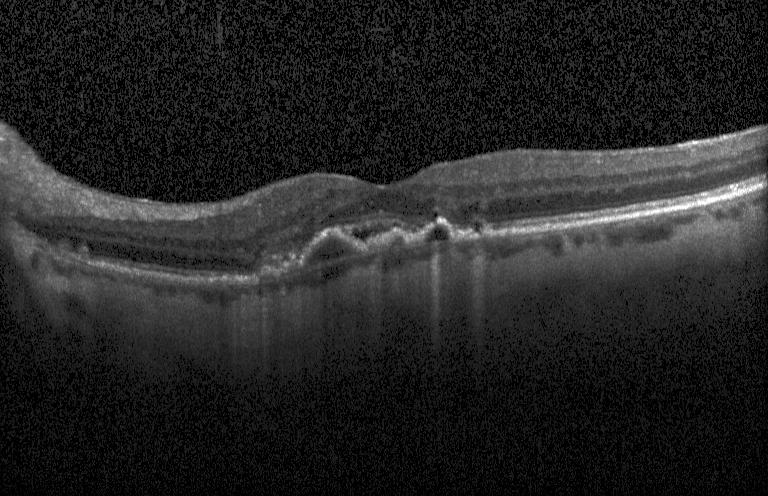 Fovea-centered. Optical coherence tomography B-scan.
The scan shows a choroidal neovascular membrane.